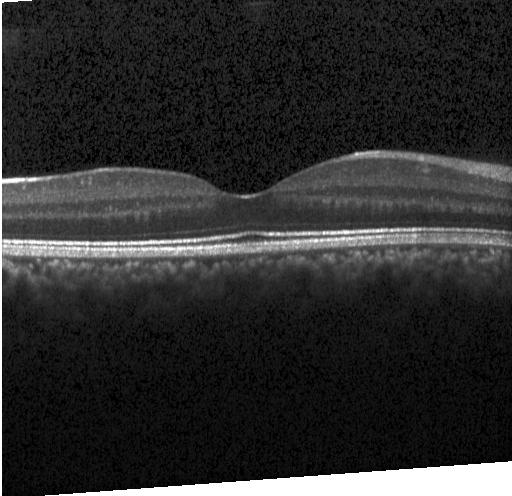

OCT B-scan, Heidelberg Spectralis OCT system
Impression: no choroidal neovascularization, diabetic macular edema, or drusen.